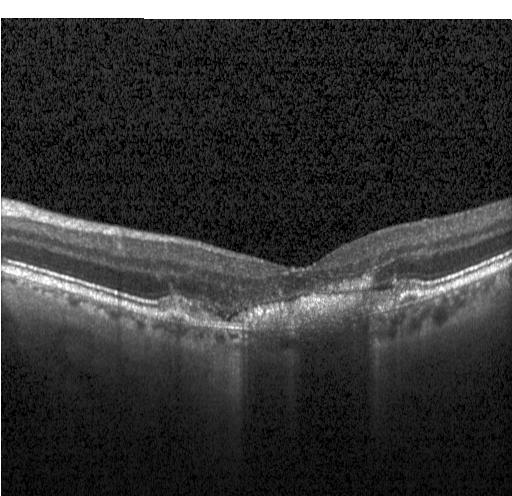
Acquired on a Heidelberg Spectralis · OCT B-scan — The scan shows choroidal neovascularization (CNV).